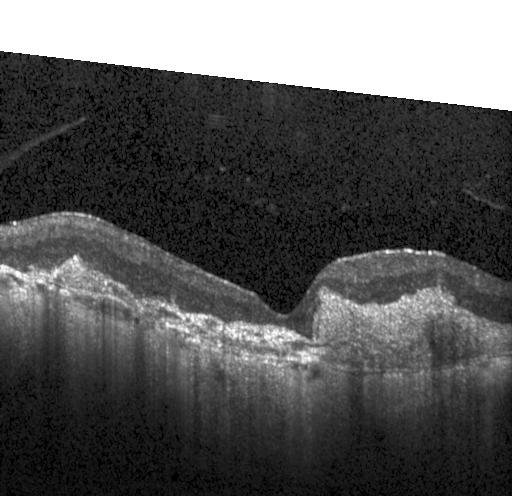

Macular OCT demonstrating a choroidal neovascular membrane.